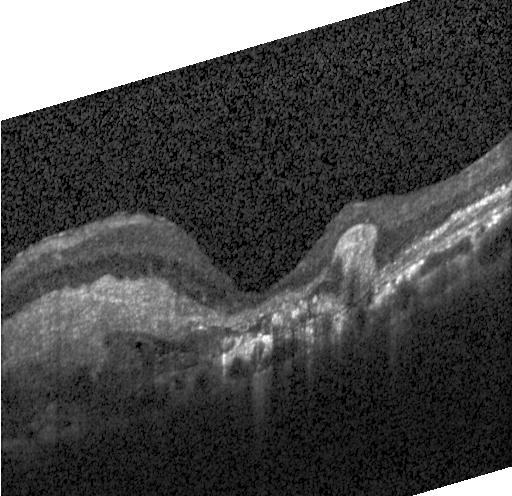

OCT scan showing a choroidal neovascular membrane.